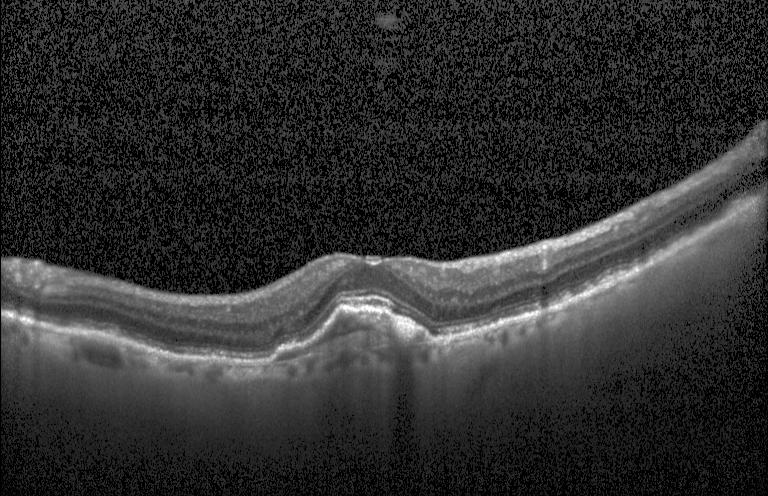 Spectral-domain optical coherence tomography. Optical coherence tomography B-scan. Heidelberg Spectralis OCT system
Assessment: a choroidal neovascular membrane.